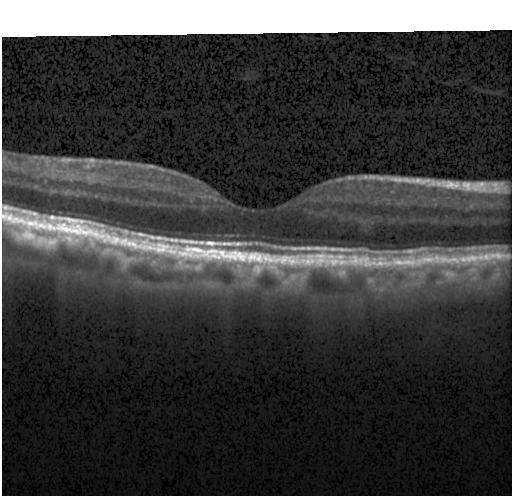 OCT scan showing no choroidal neovascularization, diabetic macular edema, or drusen.